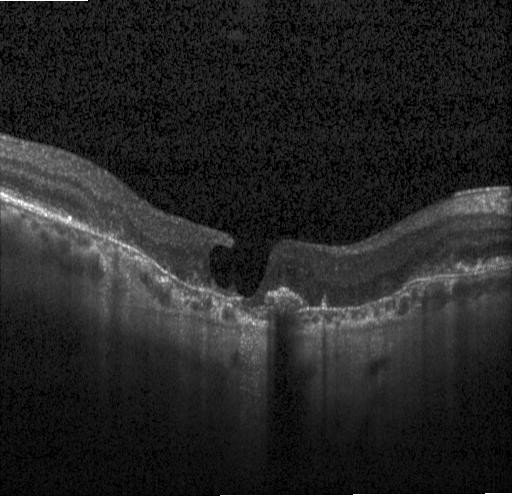
Impression: choroidal neovascularization (CNV).